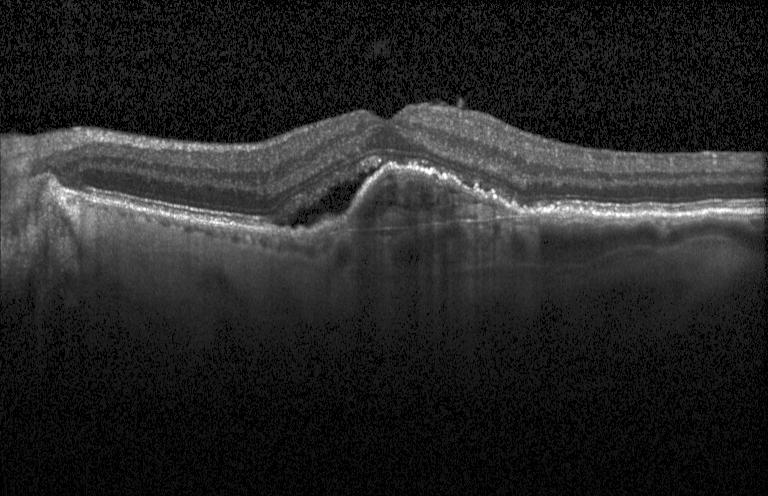 Through the macula; OCT B-scan; spectral-domain OCT; instrument: Heidelberg Spectralis. Impression: a choroidal neovascular membrane.